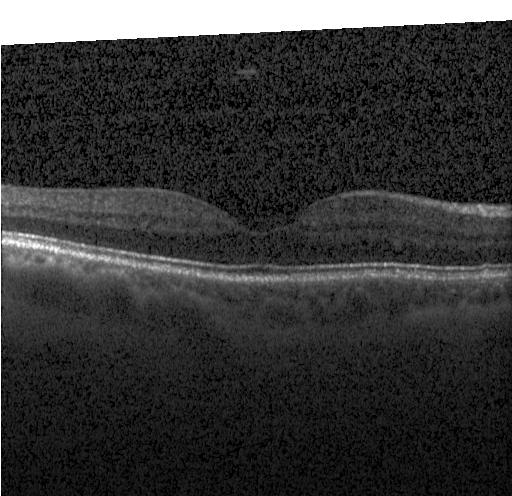 Instrument: Heidelberg Spectralis. Spectral-domain optical coherence tomography. Optical coherence tomography scan — OCT finding: no choroidal neovascularization, no diabetic macular edema, and no drusen.